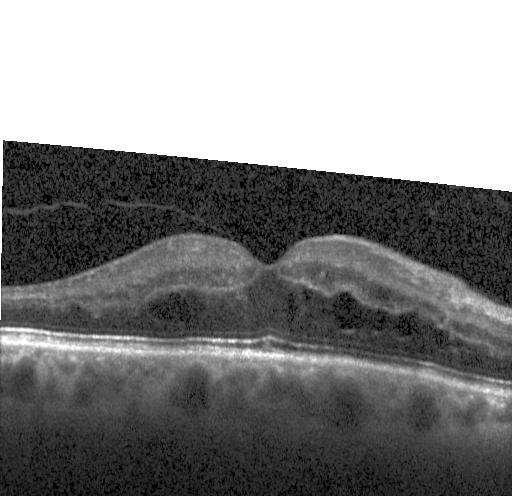
Spectral-domain OCT B-scan: diabetic macular edema.